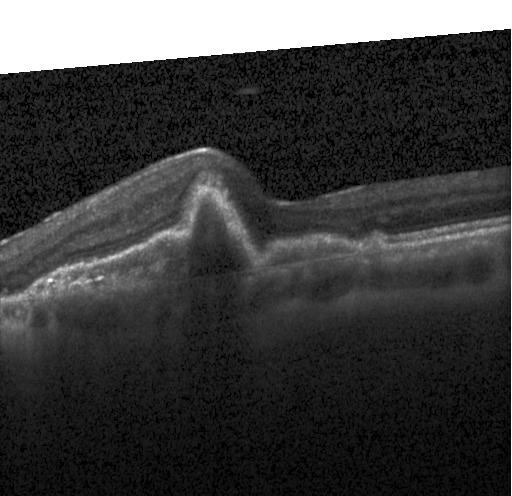
Spectral-domain OCT · optical coherence tomography scan · fovea-centered · Heidelberg Spectralis. OCT finding: a choroidal neovascular membrane.